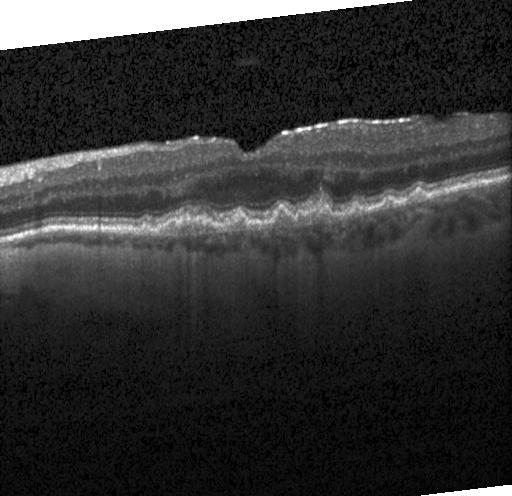 Diagnosis: sub-RPE drusenoid deposits.